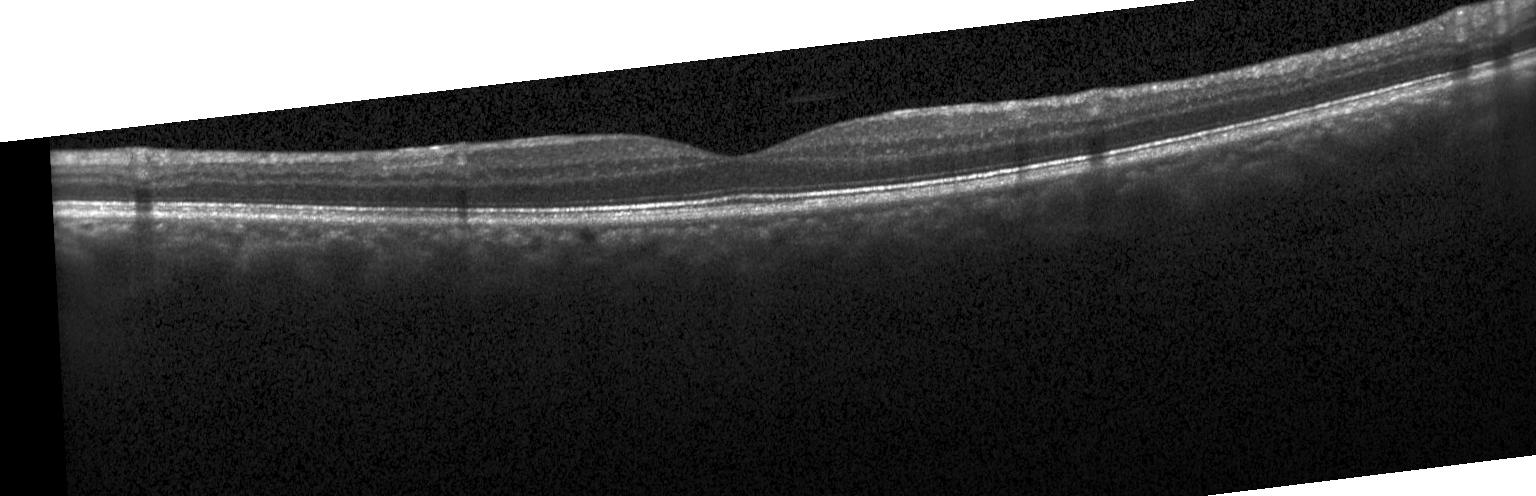

Macular OCT demonstrating no CNV, no DME, and no drusen.